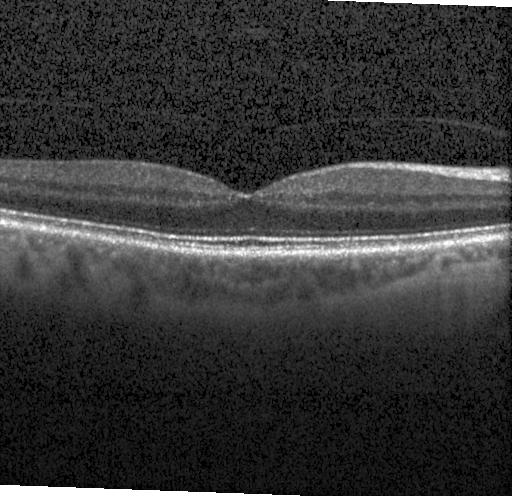 Retinal OCT cross-section; centered on the fovea; SD-OCT; Heidelberg Spectralis
Macular OCT: no choroidal neovascularization, diabetic macular edema, or drusen.